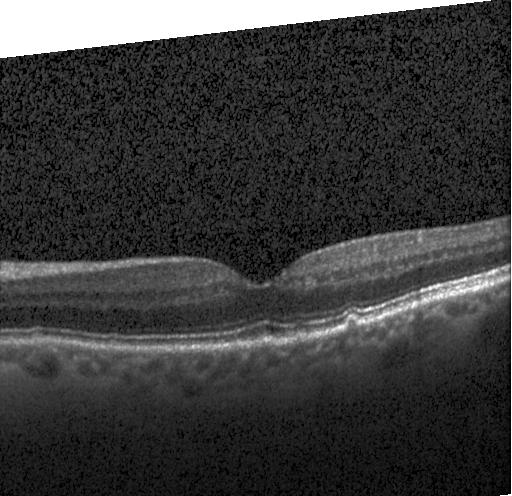 SD-OCT. Heidelberg Spectralis. OCT B-scan — Assessment: drusen.